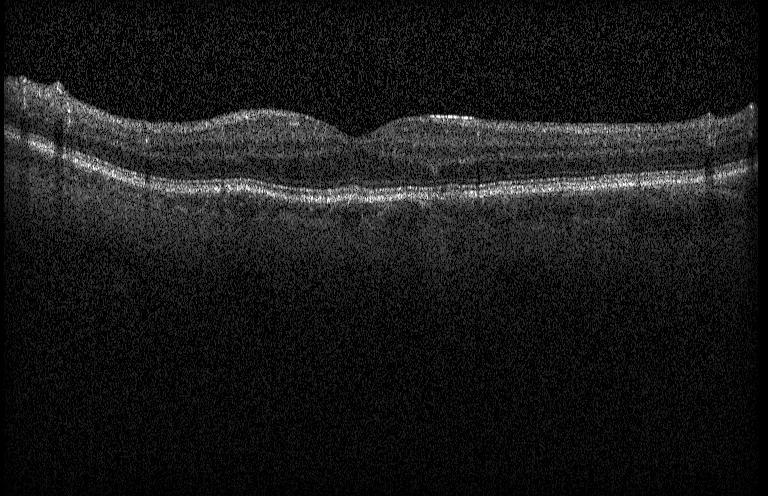

Fovea-centered · optical coherence tomography B-scan · Heidelberg Spectralis OCT system — Assessment: neither choroidal neovascularization, diabetic macular edema, nor drusen.